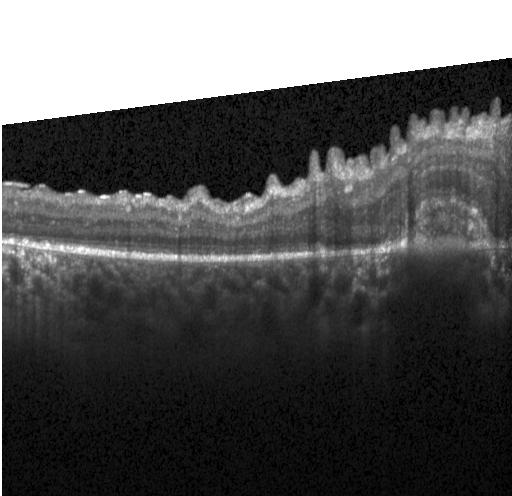

OCT line scan. Macular OCT: CNV.